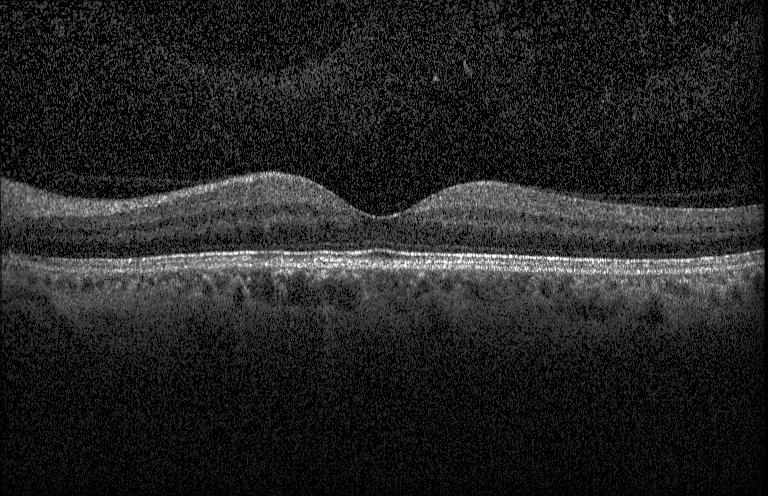

Heidelberg Spectralis OCT system · retinal OCT B-scan · spectral-domain optical coherence tomography — The scan shows no choroidal neovascularization, diabetic macular edema, or drusen.